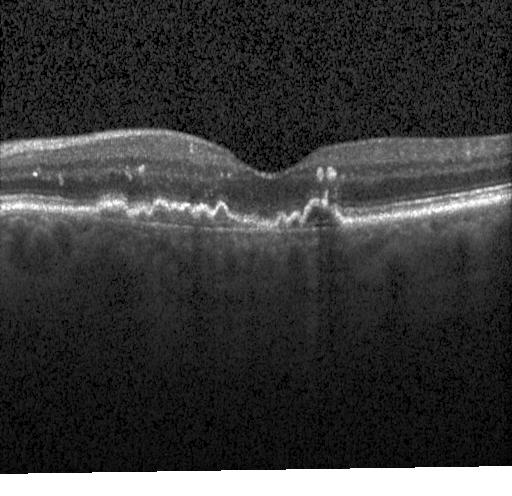
Spectral-domain optical coherence tomography, OCT line scan, through the macula
Dx: a choroidal neovascular membrane.